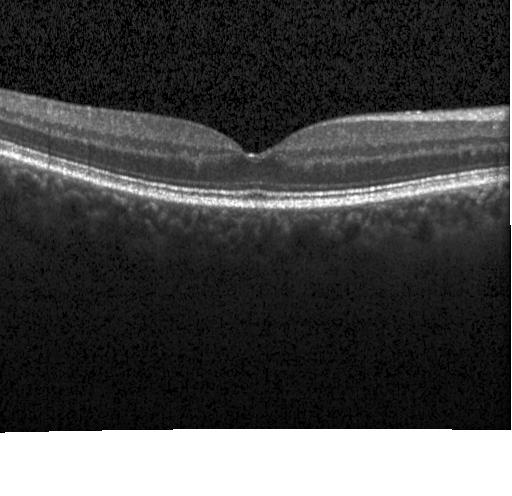
OCT line scan
Finding: no CNV, no DME, and no drusen.